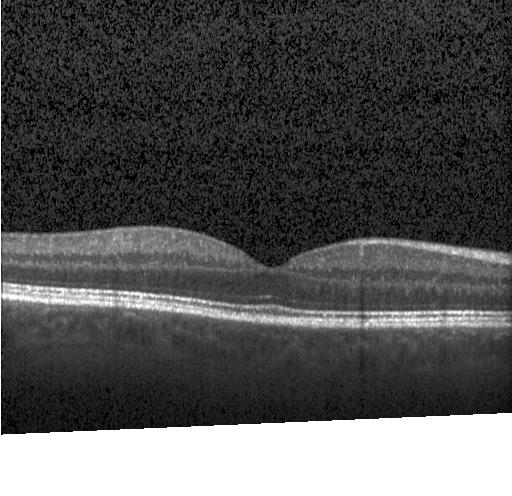

Macular OCT: neither CNV, DME, nor drusen.